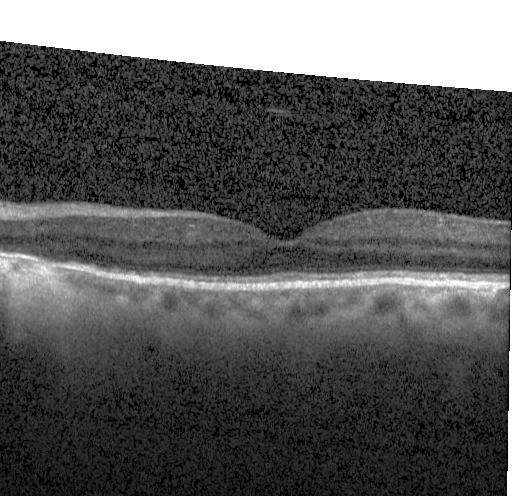

Impression: neither choroidal neovascularization, diabetic macular edema, nor drusen.